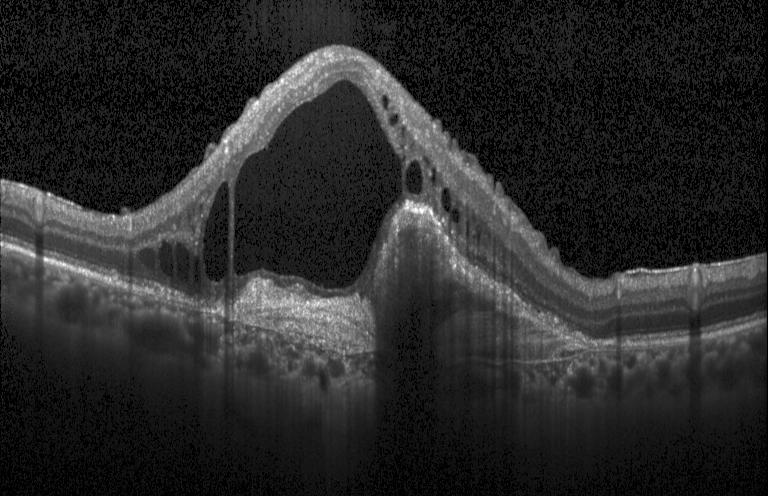 Retinal OCT B-scan. Heidelberg Spectralis. Through the macula. Spectral-domain OCT. Impression: choroidal neovascularization (CNV).